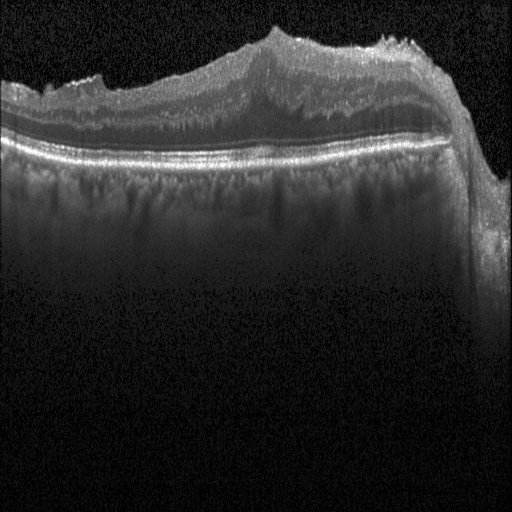
OCT B-scan — Impression: diabetic macular edema.